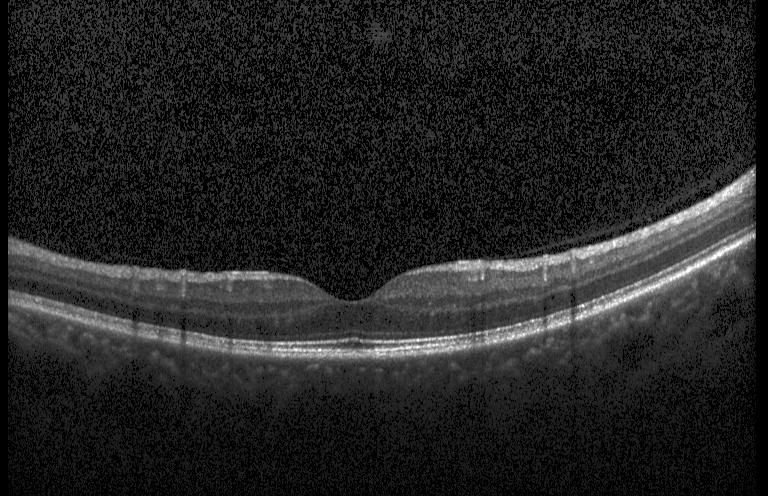
SD-OCT · Heidelberg Spectralis · OCT line scan. Diagnosis: no choroidal neovascularization, no diabetic macular edema, and no drusen.